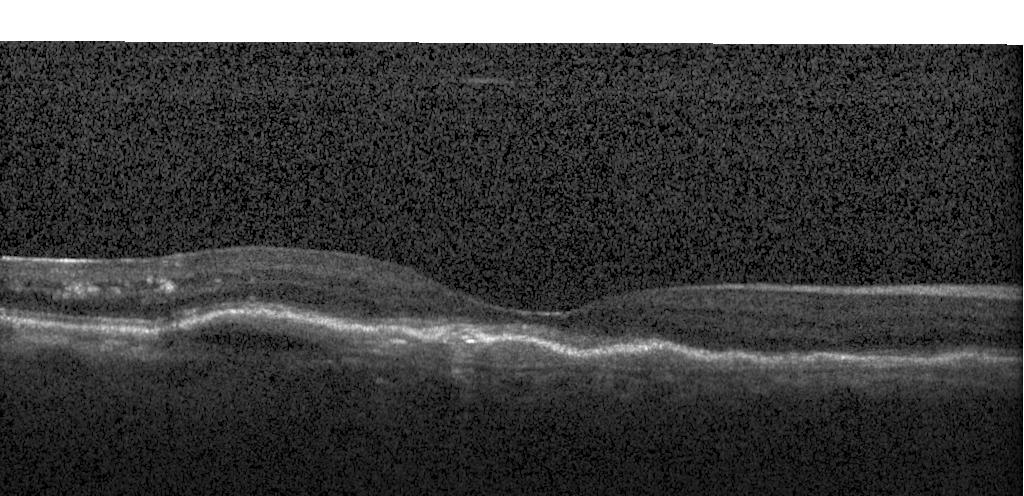

Centered on the fovea. Spectral-domain OCT. OCT B-scan. Heidelberg Spectralis OCT system
Dx: a choroidal neovascular membrane.